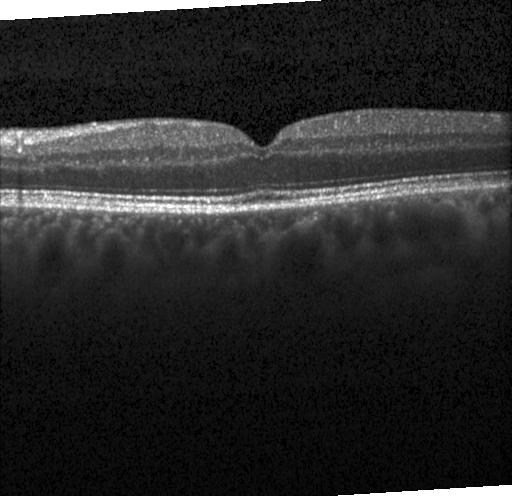

Through the macula, optical coherence tomography B-scan, acquired on a Heidelberg Spectralis, spectral-domain optical coherence tomography
Assessment: no choroidal neovascularization, diabetic macular edema, or drusen.